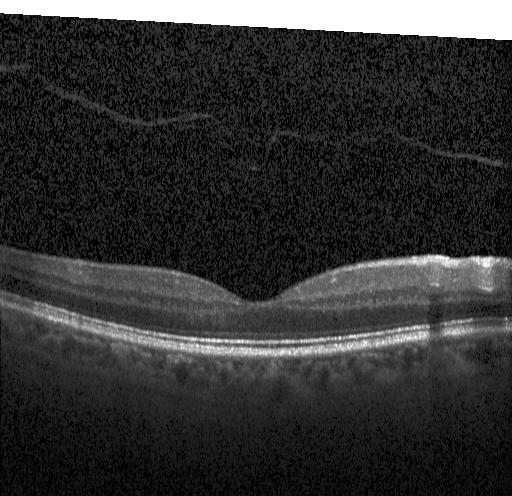

OCT B-scan.
The scan shows neither CNV, DME, nor drusen.